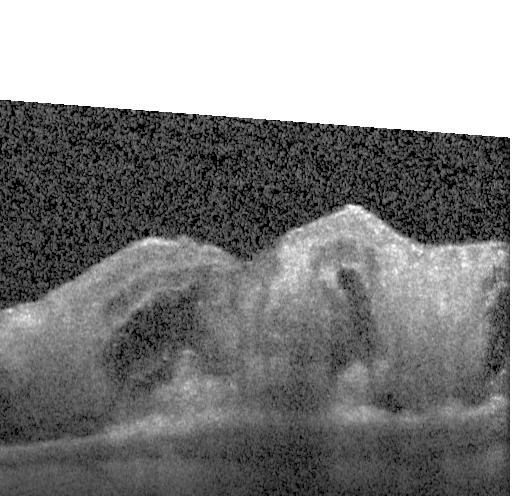
Dx: a choroidal neovascular membrane.